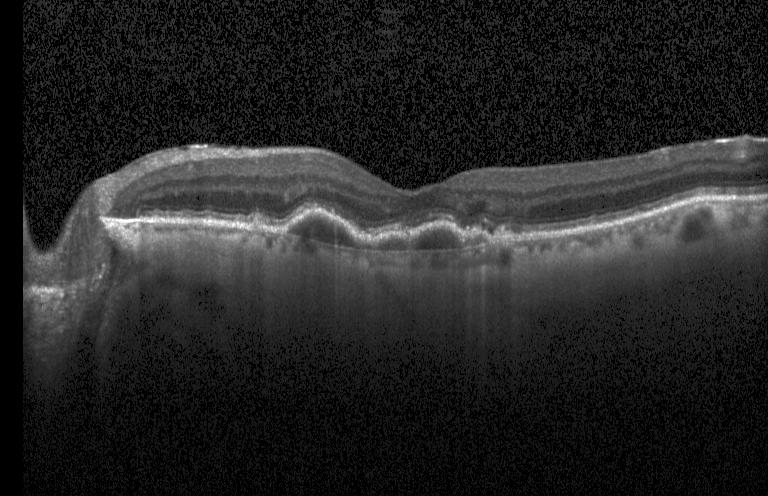

Retinal OCT B-scan. Finding: CNV.